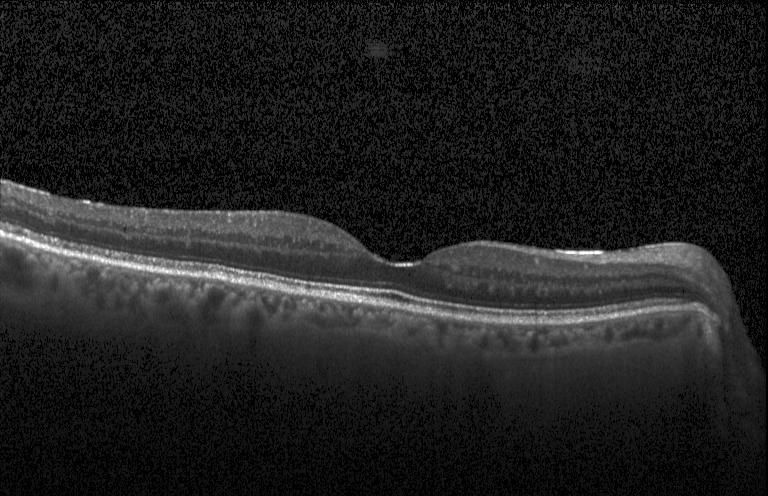 Spectral-domain OCT, centered on the fovea, retinal OCT B-scan
Diagnosis: no choroidal neovascularization, no diabetic macular edema, and no drusen.